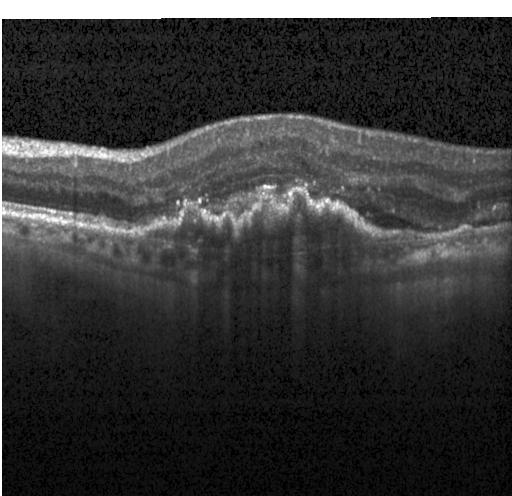 Finding: a choroidal neovascular membrane.